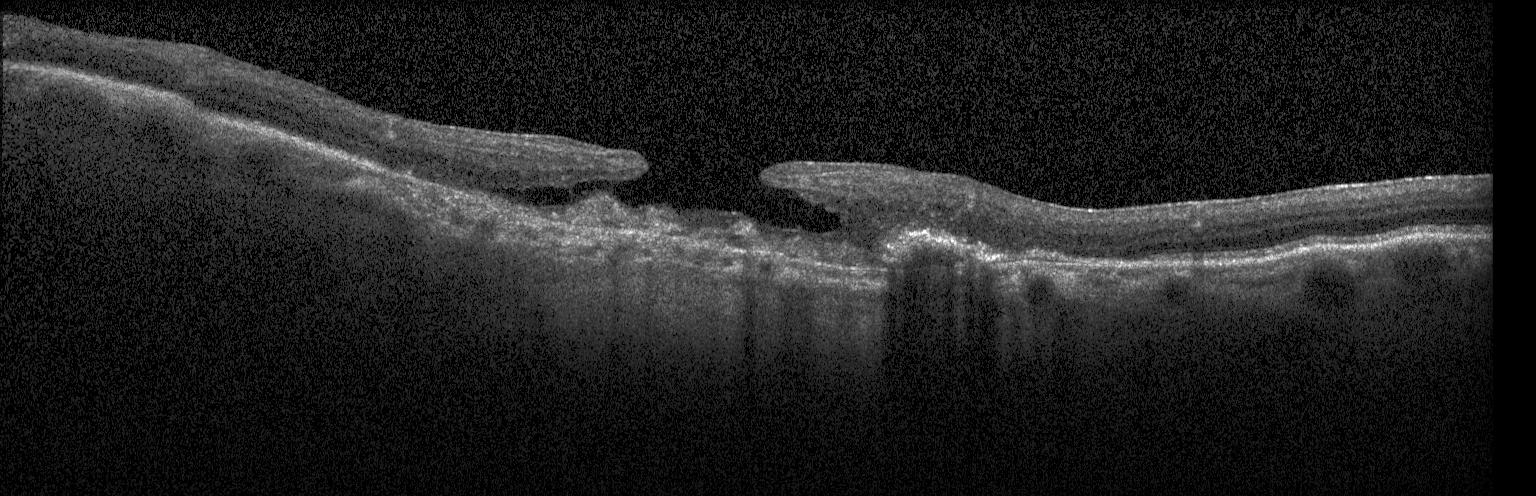 OCT B-scan — Impression: a choroidal neovascular membrane.